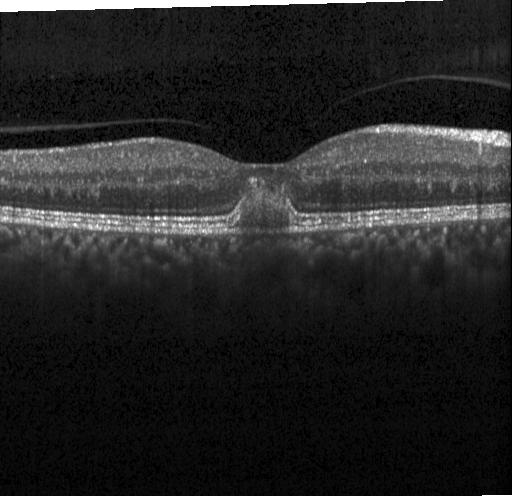

Instrument: Heidelberg Spectralis; optical coherence tomography scan.
Impression: choroidal neovascularization.